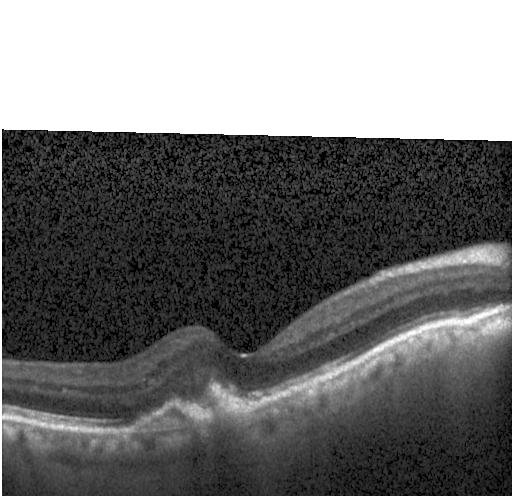
Diagnosis: choroidal neovascularization.